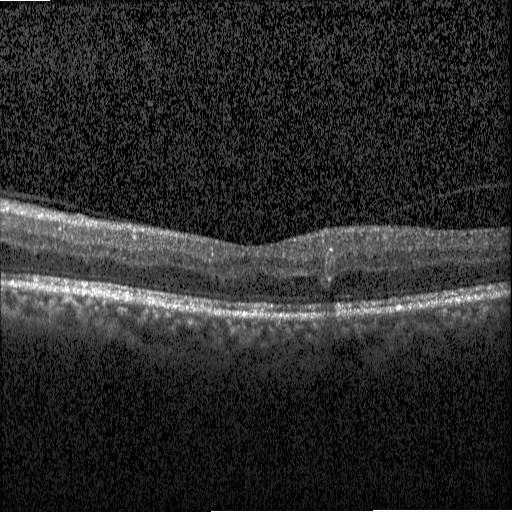 OCT line scan; acquired on a Heidelberg Spectralis; horizontal scan through the fovea.
Impression: diabetic macular edema (DME).